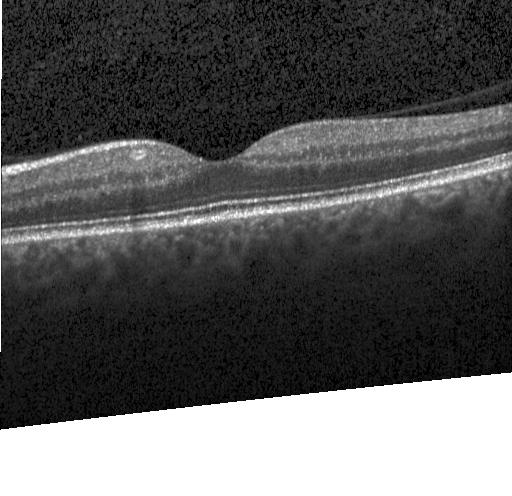

Finding: no choroidal neovascularization, no diabetic macular edema, and no drusen.